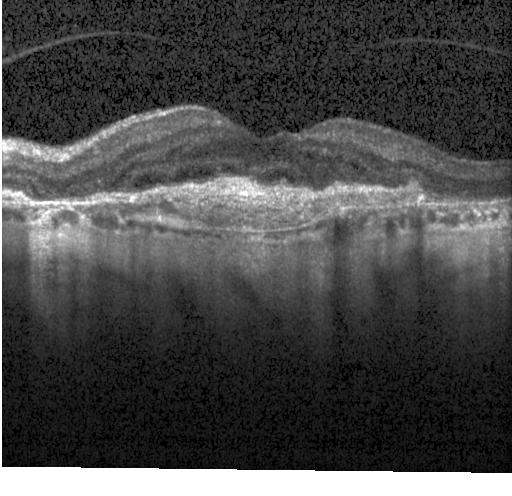 Optical coherence tomography scan, through the macula, acquired on a Heidelberg Spectralis
Diagnosis: CNV.